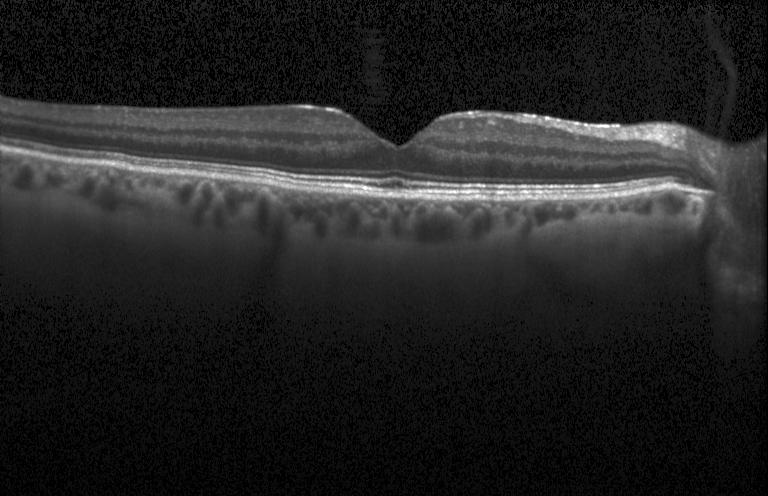
Macular scan. Heidelberg Spectralis OCT system. Optical coherence tomography B-scan. SD-OCT
Assessment: no CNV, DME, or drusen.